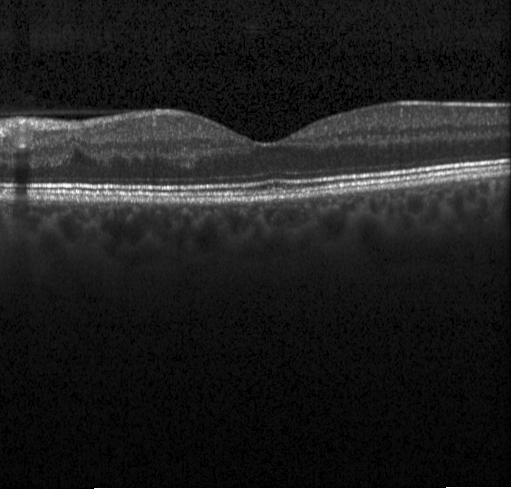

Optical coherence tomography B-scan, Heidelberg Spectralis OCT system, through the macula
Assessment: neither choroidal neovascularization, diabetic macular edema, nor drusen.